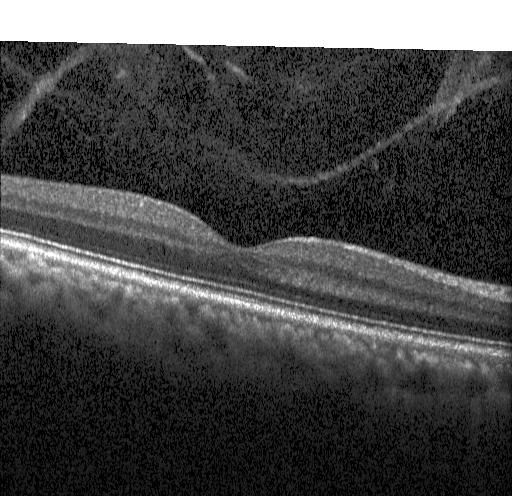

Retinal OCT B-scan · spectral-domain OCT · Heidelberg Spectralis OCT system — The scan shows no CNV, no DME, and no drusen.